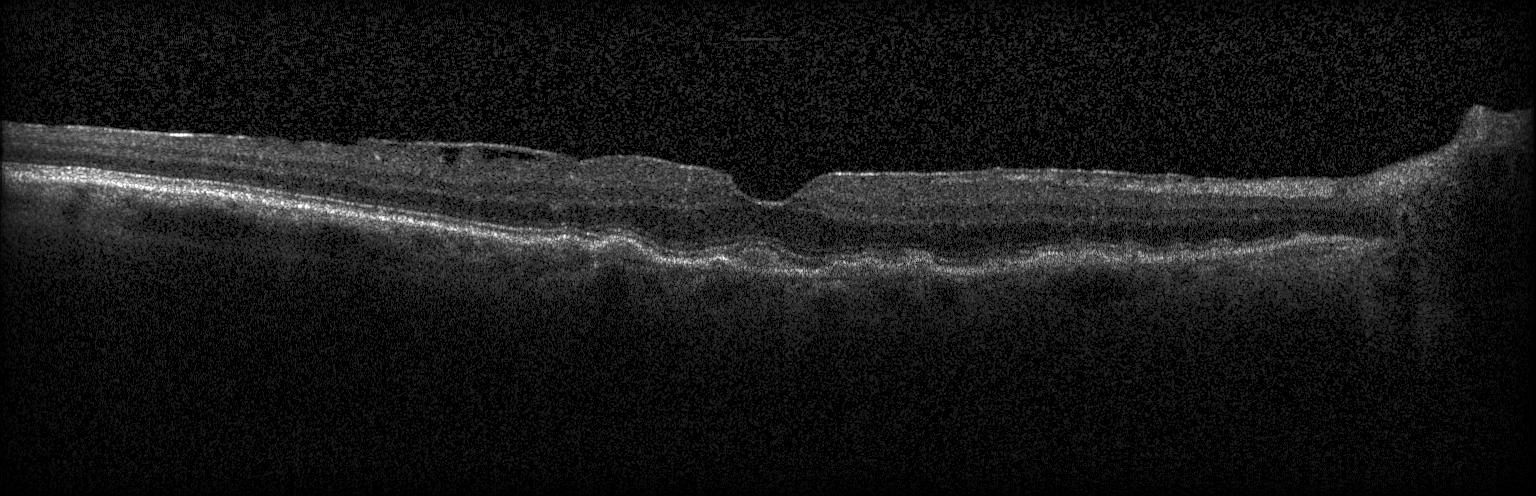

Finding: drusen.